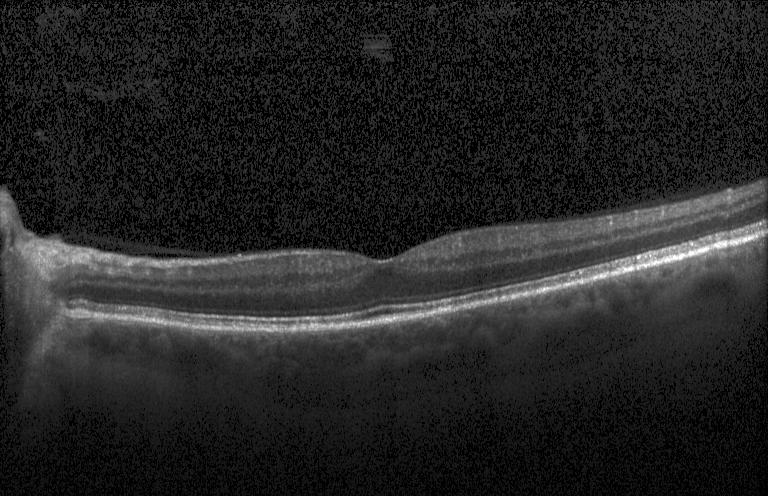 Impression: no choroidal neovascularization, diabetic macular edema, or drusen.